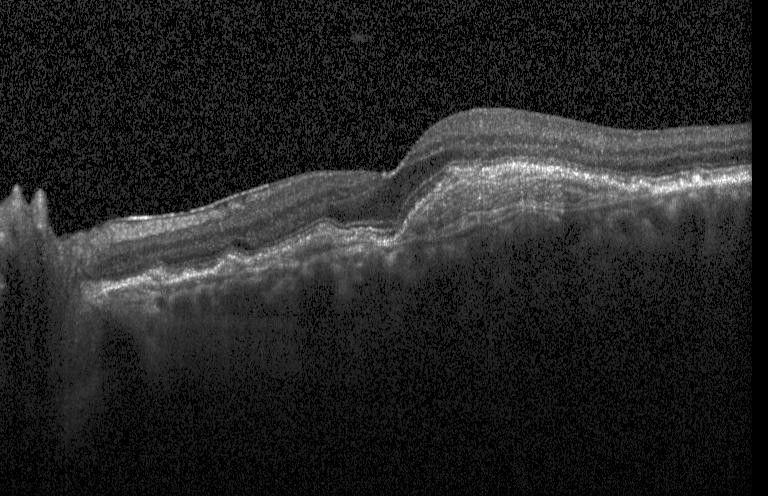

Optical coherence tomography scan
Dx: choroidal neovascularization (CNV).